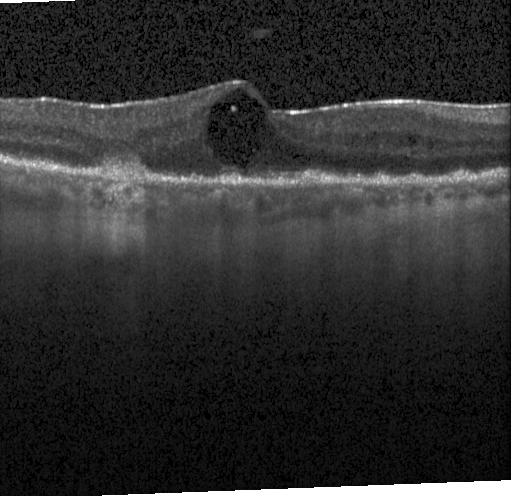 OCT B-scan, instrument: Heidelberg Spectralis. Finding: a choroidal neovascular membrane.